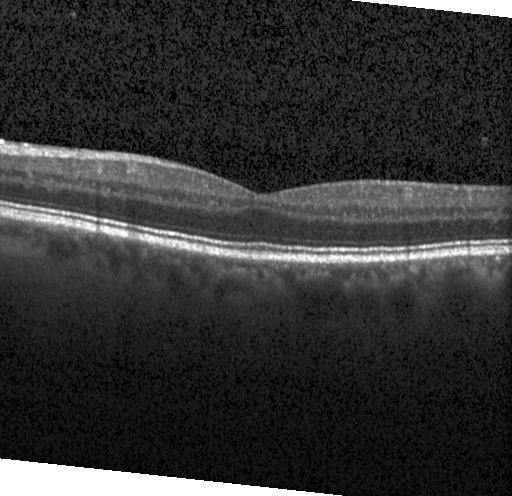

Heidelberg Spectralis OCT system. Retinal OCT cross-section. Through the macula
Finding: no evidence of choroidal neovascularization, diabetic macular edema, or drusen.